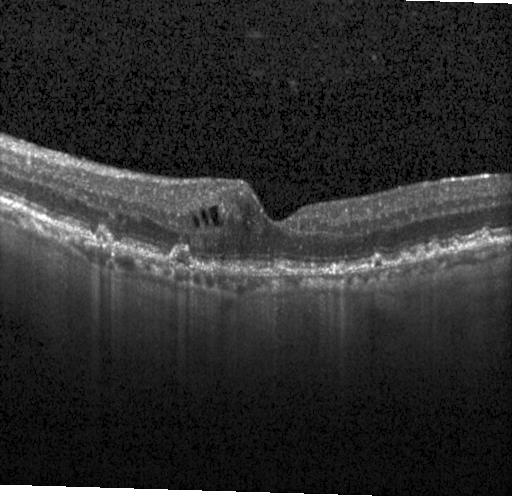
The scan shows a choroidal neovascular membrane.